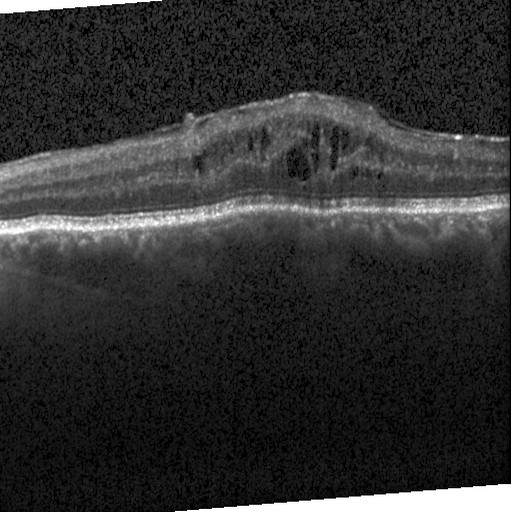
Assessment: diabetic macular edema (DME).